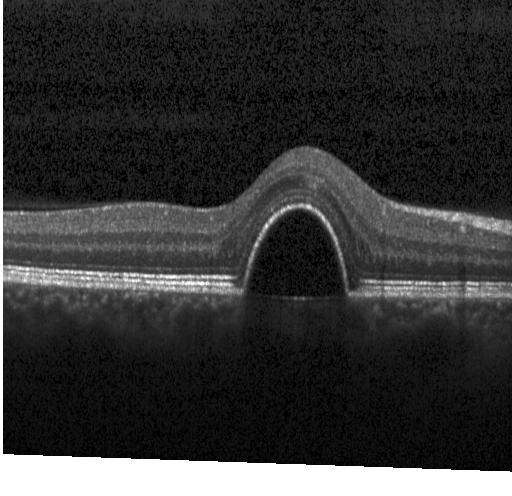 Horizontal scan through the fovea, OCT line scan, spectral-domain OCT.
CNV.